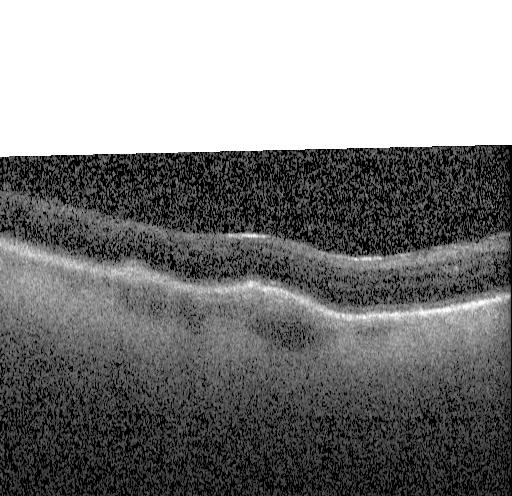
Horizontal scan through the fovea; optical coherence tomography scan; spectral-domain OCT; instrument: Heidelberg Spectralis. This B-scan demonstrates choroidal neovascularization (CNV).